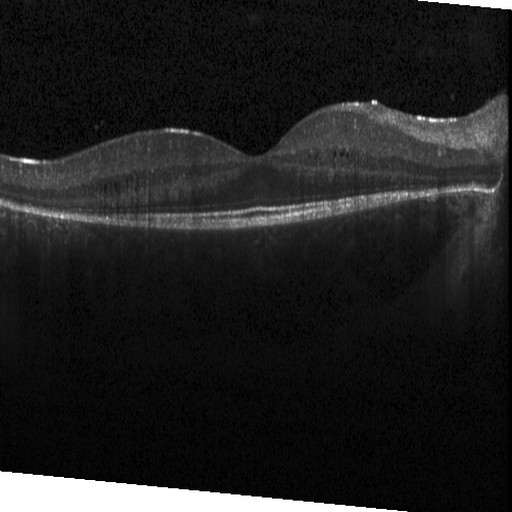 Heidelberg Spectralis OCT system; centered on the fovea; optical coherence tomography B-scan
Assessment: diabetic macular edema.